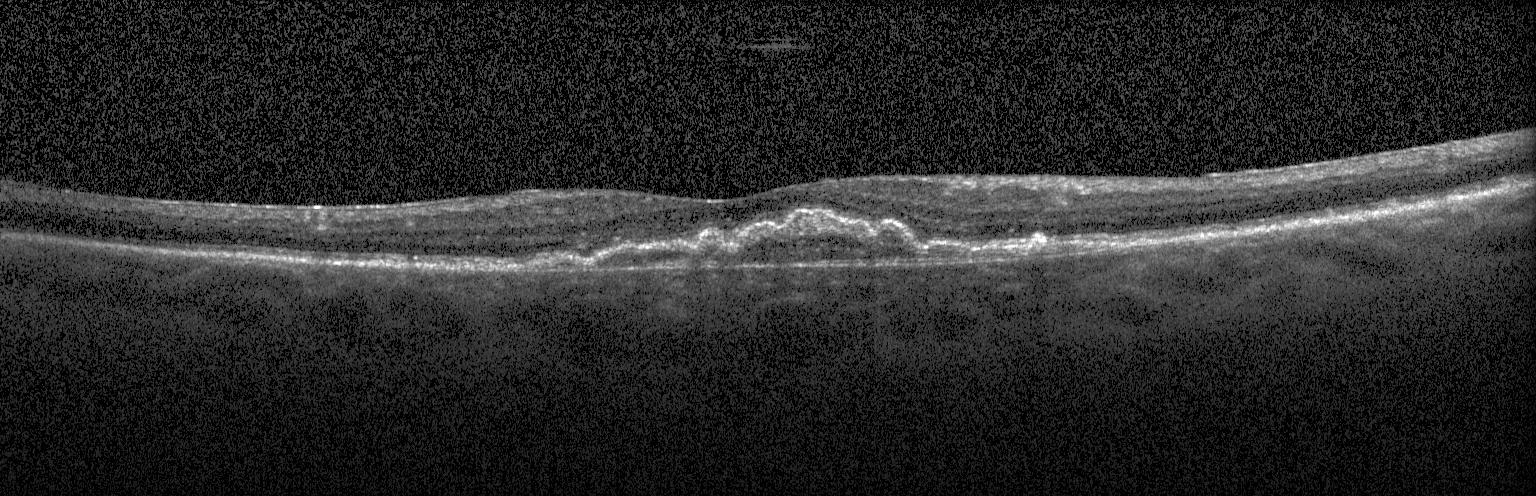 Diagnosis: a choroidal neovascular membrane.